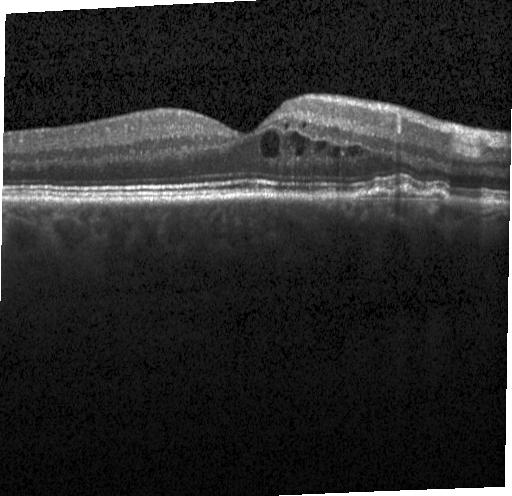

Finding: choroidal neovascularization.